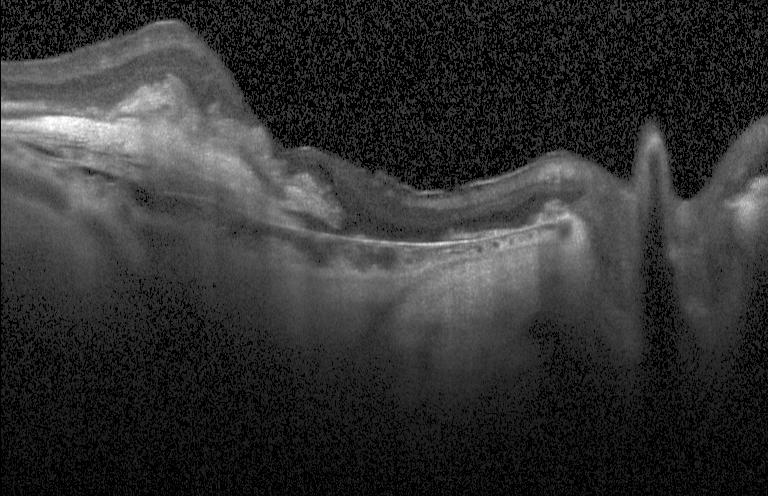
Spectral-domain optical coherence tomography · optical coherence tomography scan · instrument: Heidelberg Spectralis. This B-scan demonstrates a choroidal neovascular membrane.